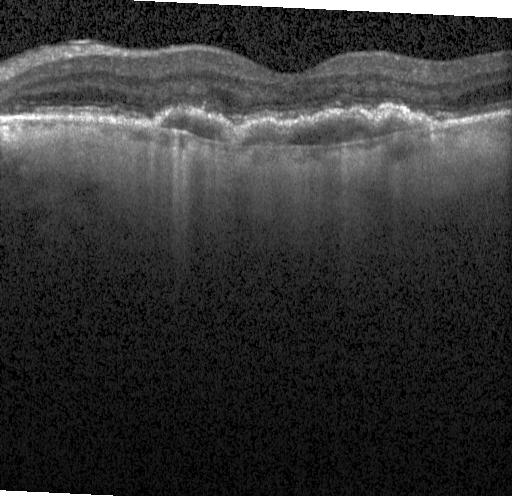
Through the macula · optical coherence tomography B-scan.
Finding: a choroidal neovascular membrane.